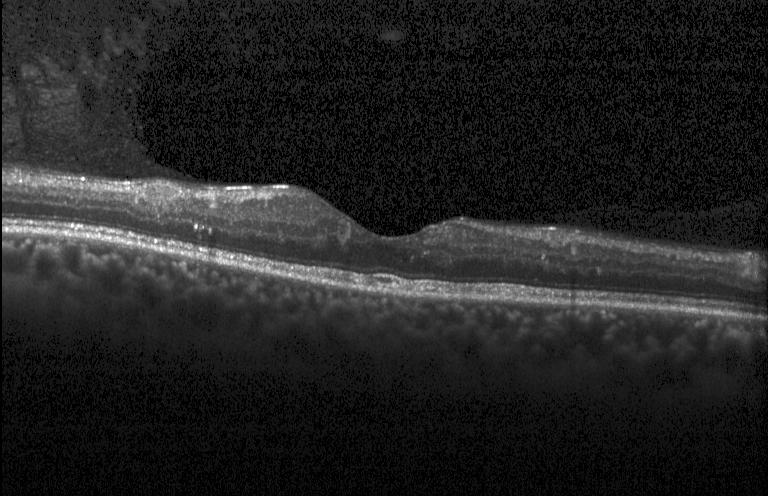
Finding: diabetic macular edema (DME).